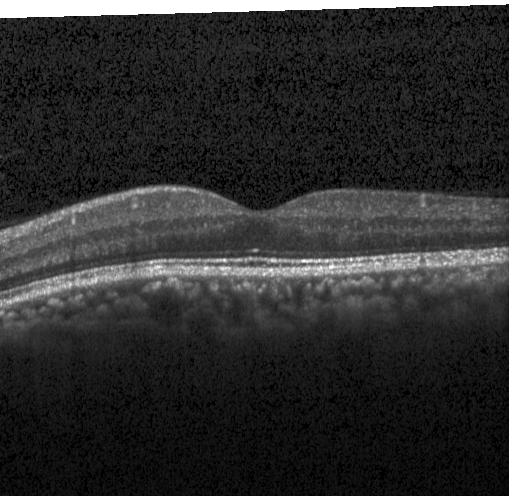 Spectral-domain OCT B-scan: neither CNV, DME, nor drusen.